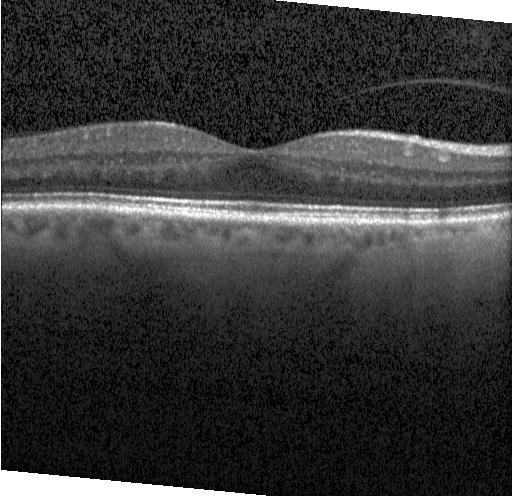
Fovea-centered. Heidelberg Spectralis. Spectral-domain optical coherence tomography. Optical coherence tomography B-scan.
The scan shows neither choroidal neovascularization, diabetic macular edema, nor drusen.